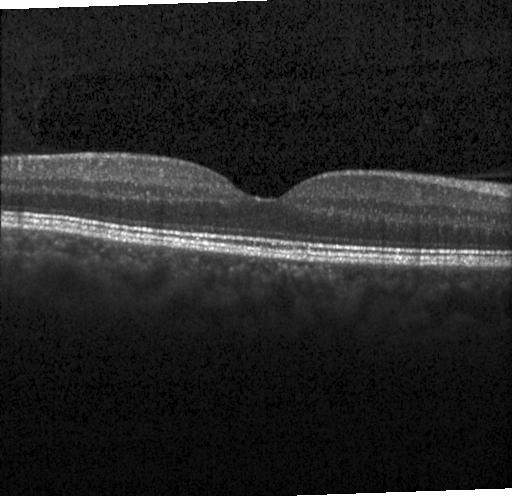

Optical coherence tomography B-scan.
Finding: neither CNV, DME, nor drusen.